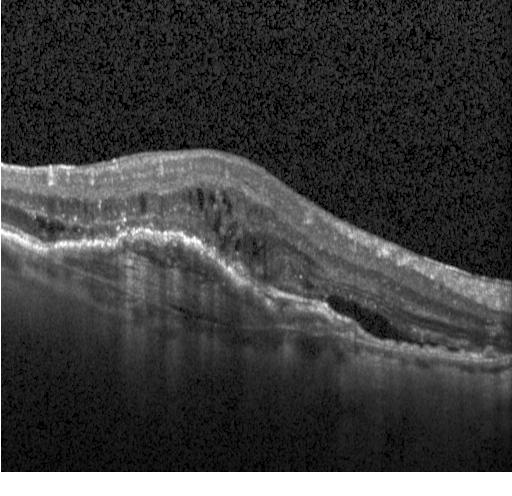 OCT line scan, spectral-domain optical coherence tomography, macular scan, Heidelberg Spectralis
The scan shows choroidal neovascularization.